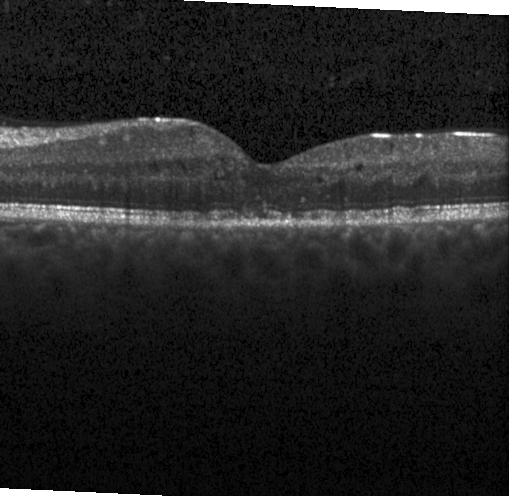
Optical coherence tomography scan — Impression: DME.